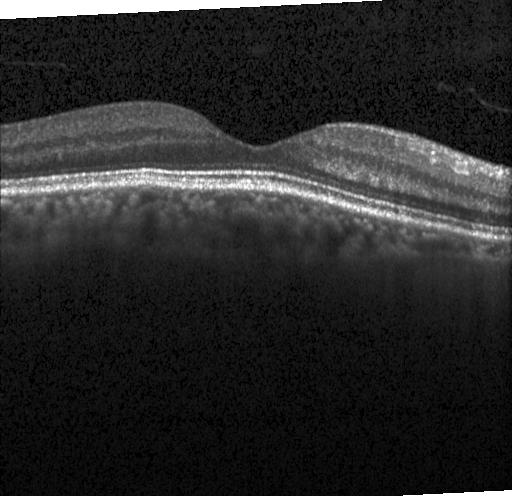
Assessment: no CNV, no DME, and no drusen.